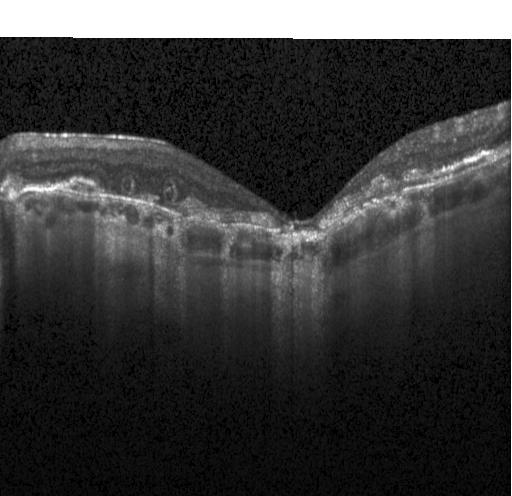 Assessment: CNV.